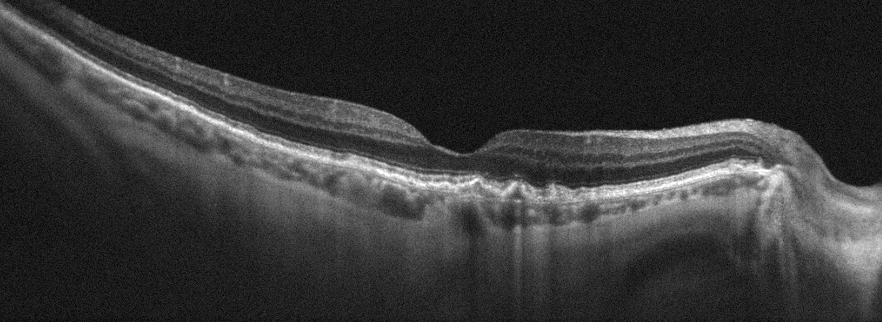

Right eye, optical coherence tomography B-scan
This B-scan demonstrates age-related macular degeneration (AMD).